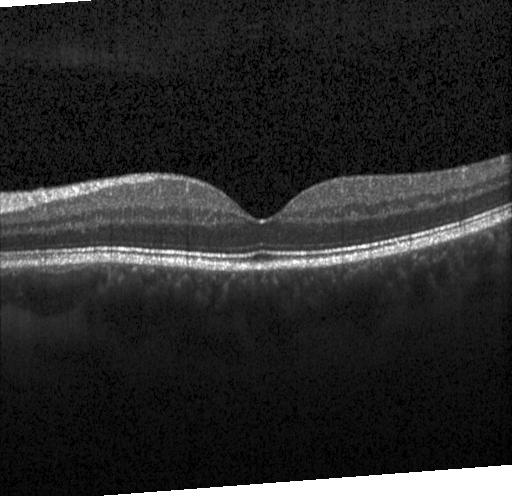 OCT scan showing no CNV, DME, or drusen.